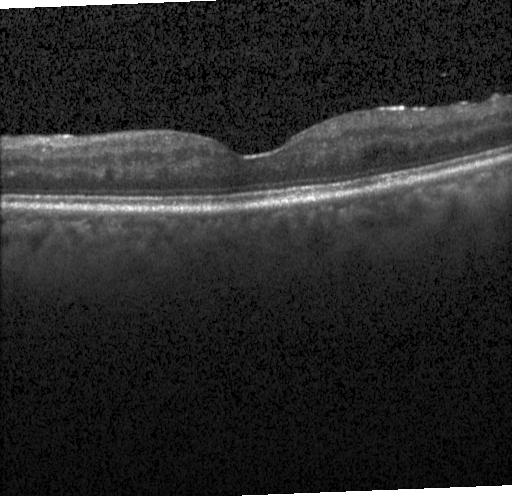
Acquired on a Heidelberg Spectralis · retinal OCT cross-section · macular scan · spectral-domain optical coherence tomography. This B-scan demonstrates no evidence of CNV, DME, or drusen.